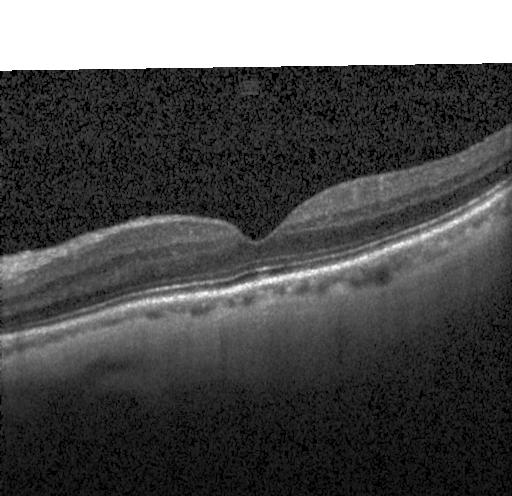 Through the macula · optical coherence tomography B-scan · Heidelberg Spectralis OCT system.
OCT finding: no choroidal neovascularization, no diabetic macular edema, and no drusen.